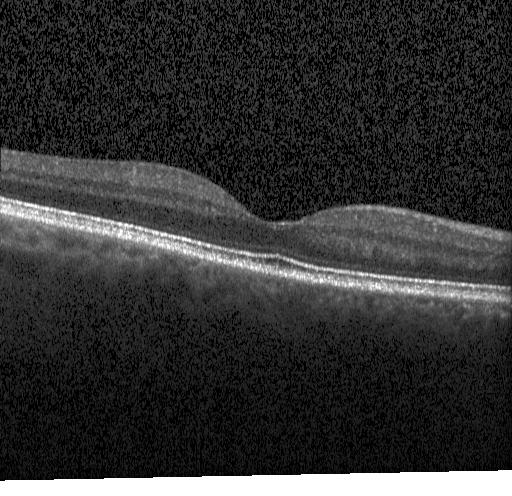
Retinal OCT B-scan. Horizontal scan through the fovea. Heidelberg Spectralis OCT system. Spectral-domain OCT — Diagnosis: no evidence of choroidal neovascularization, diabetic macular edema, or drusen.